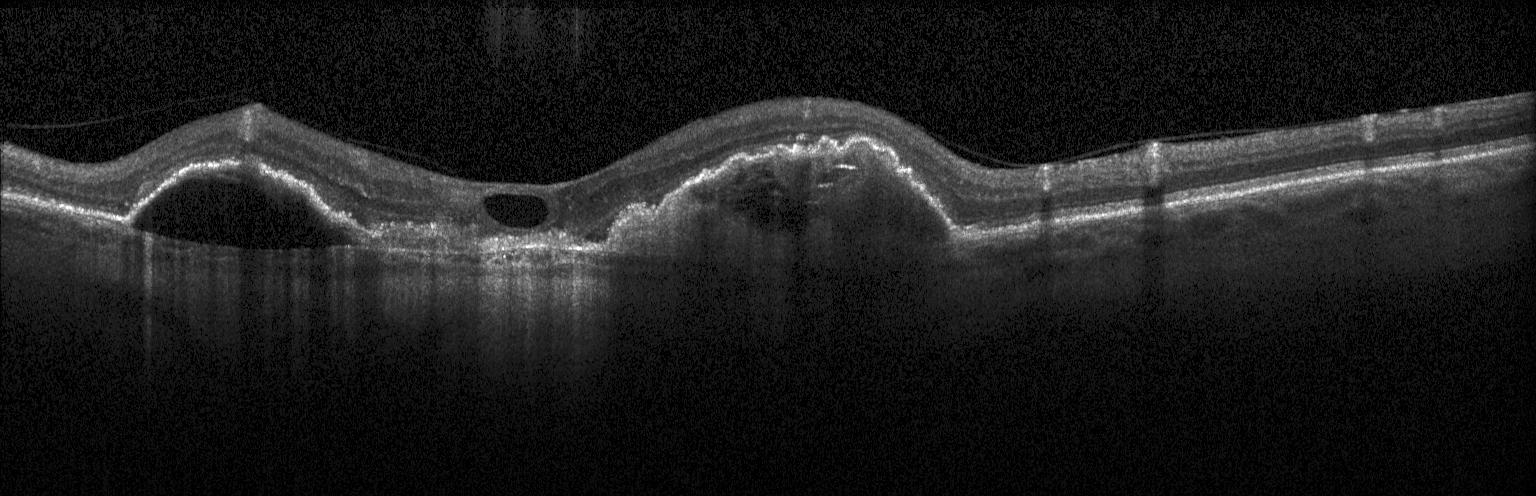
Diagnosis: a choroidal neovascular membrane.